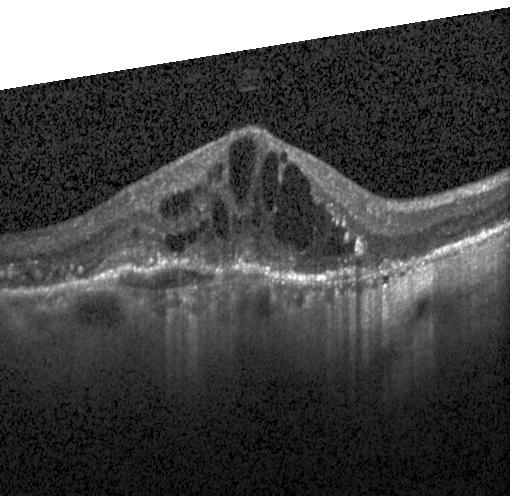

Retinal OCT cross-section, SD-OCT
The scan shows CNV.